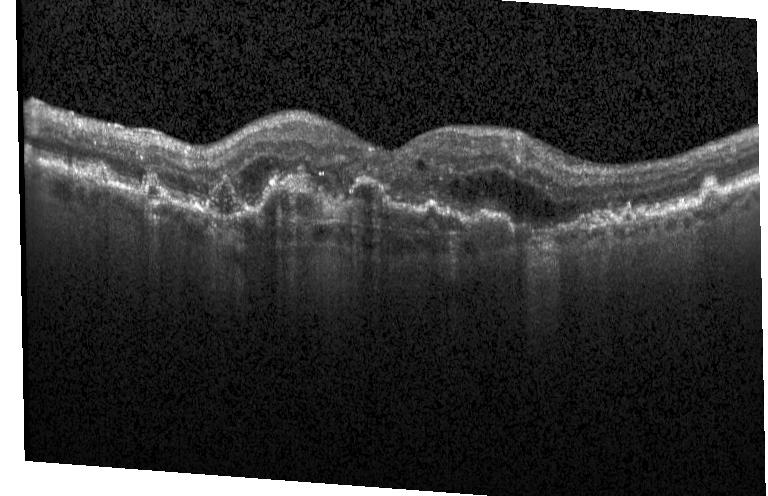 Heidelberg Spectralis · spectral-domain optical coherence tomography · through the macula · optical coherence tomography scan
Impression: choroidal neovascularization.